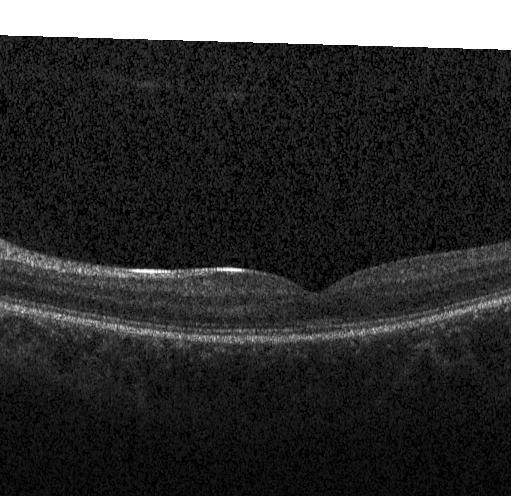

Dx: neither CNV, DME, nor drusen.